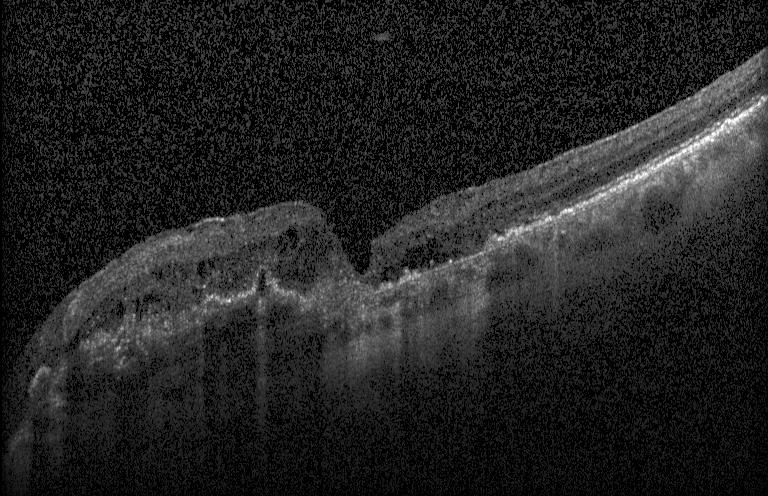

Retinal OCT cross-section
The scan shows choroidal neovascularization (CNV).